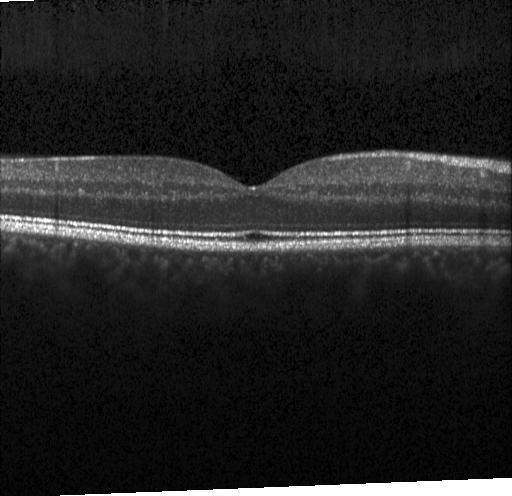 Diagnosis: no choroidal neovascularization, diabetic macular edema, or drusen.